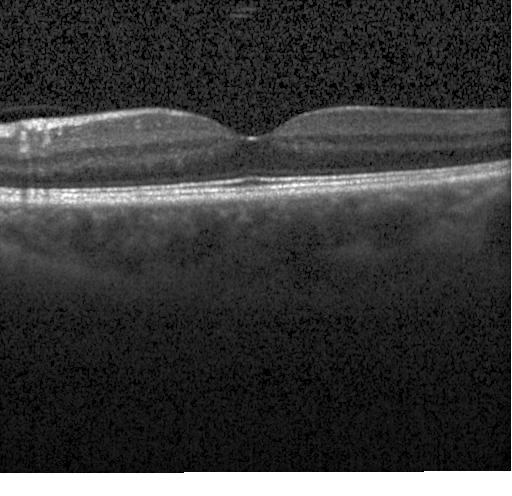
Optical coherence tomography scan, spectral-domain OCT — OCT finding: neither choroidal neovascularization, diabetic macular edema, nor drusen.